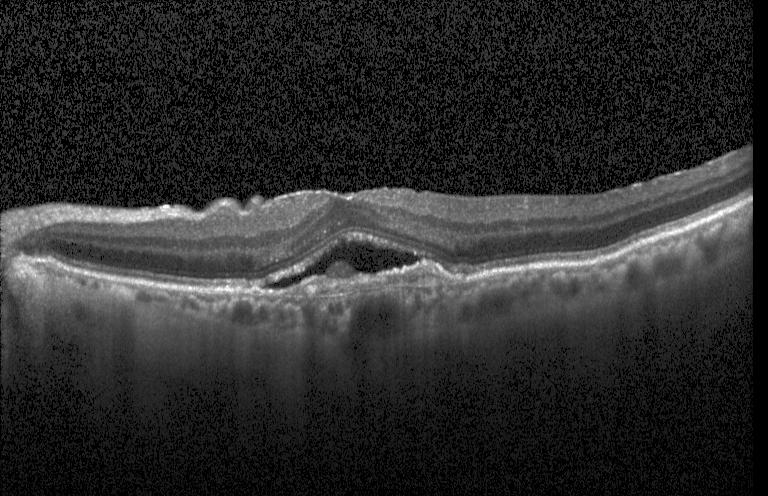
Acquired on a Heidelberg Spectralis; SD-OCT; retinal OCT B-scan. Assessment: a choroidal neovascular membrane.